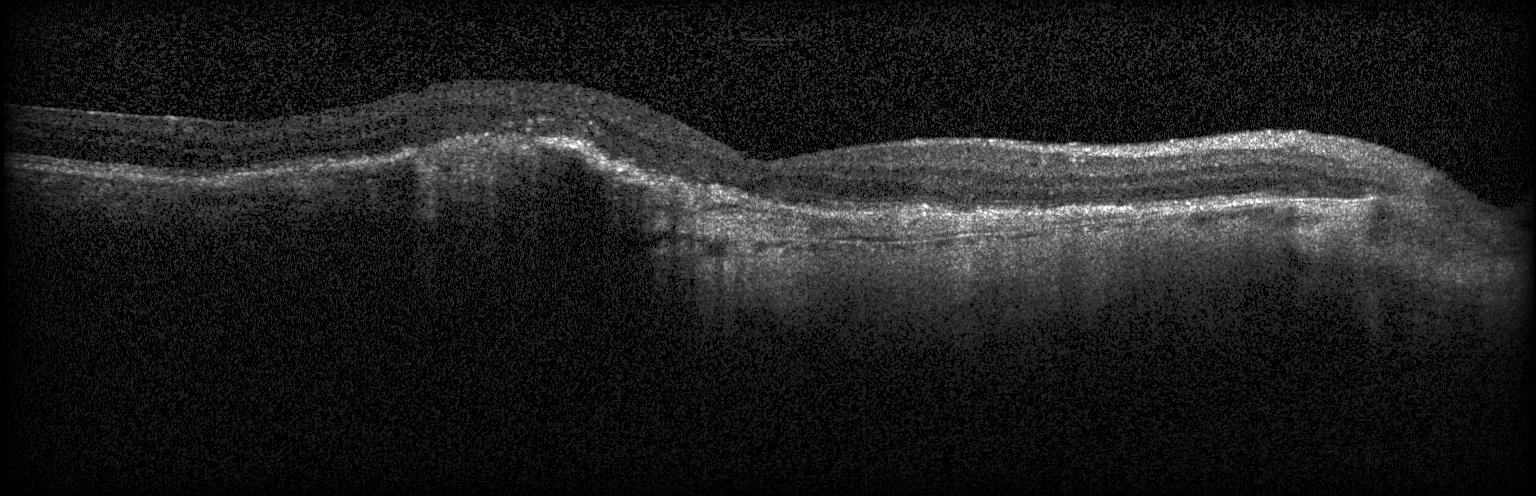
A choroidal neovascular membrane.